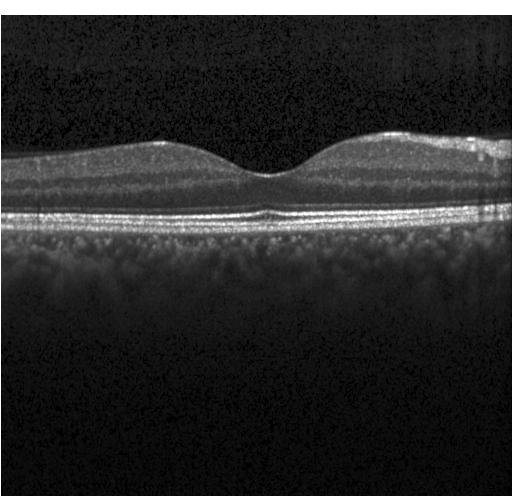

Optical coherence tomography B-scan.
Diagnosis: no CNV, no DME, and no drusen.